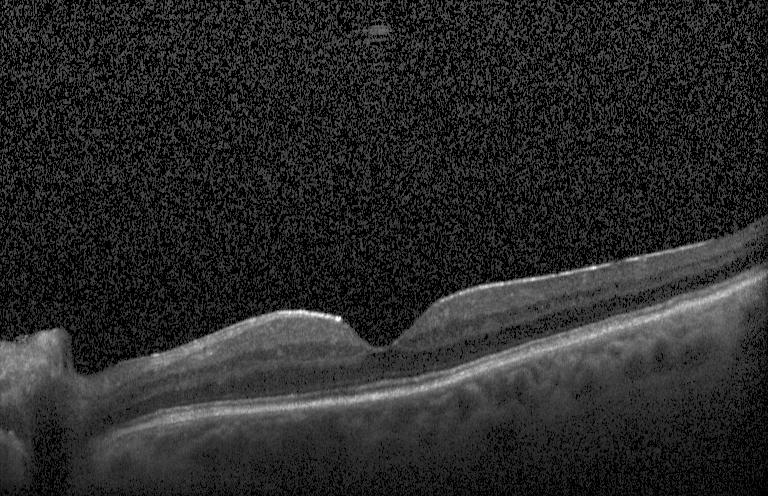
SD-OCT · retinal OCT cross-section · horizontal scan through the fovea
Impression: no choroidal neovascularization, diabetic macular edema, or drusen.